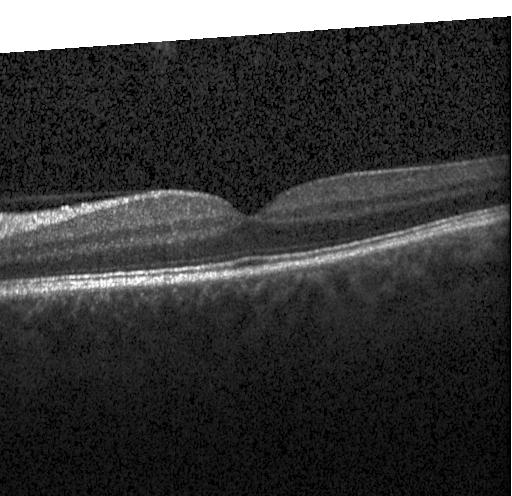
Spectral-domain OCT; retinal OCT B-scan; macular scan.
The scan shows no evidence of choroidal neovascularization, diabetic macular edema, or drusen.